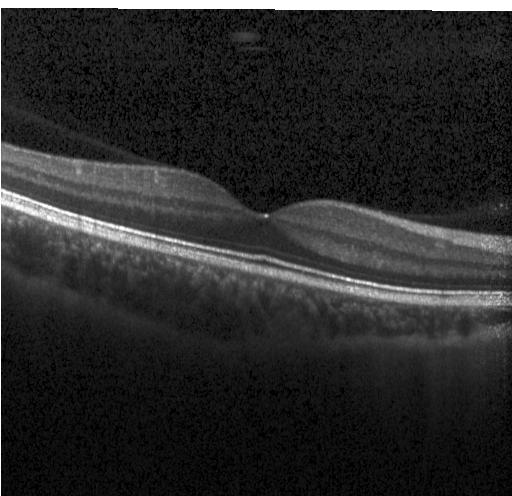 OCT line scan — This B-scan demonstrates no evidence of choroidal neovascularization, diabetic macular edema, or drusen.